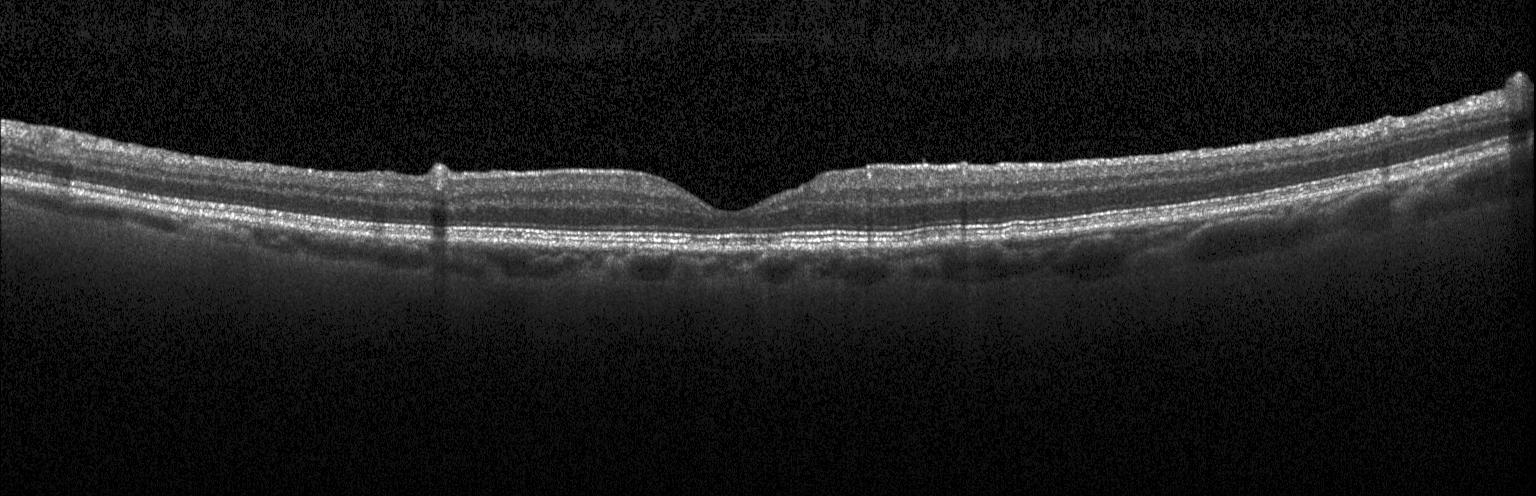
Optical coherence tomography B-scan, macular scan, SD-OCT
The scan shows no choroidal neovascularization, diabetic macular edema, or drusen.